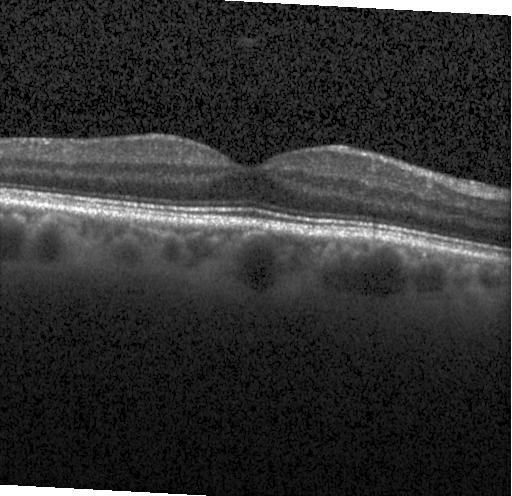

Diagnosis: no CNV, DME, or drusen.